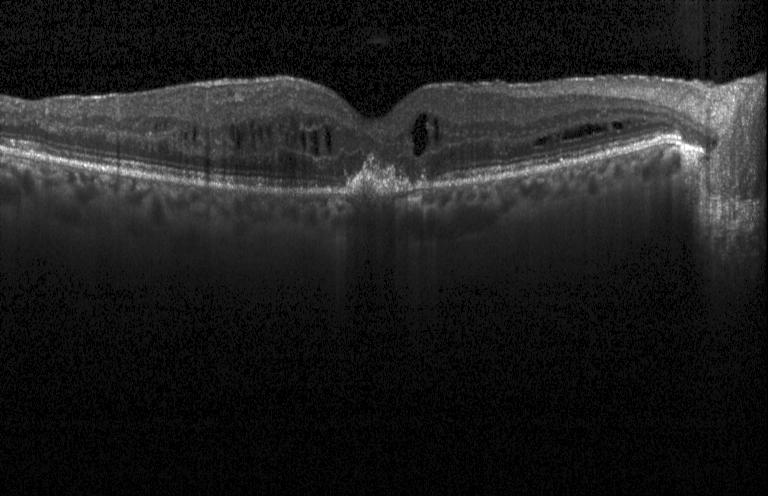 Retinal OCT B-scan, instrument: Heidelberg Spectralis.
Impression: sub-RPE drusenoid deposits.